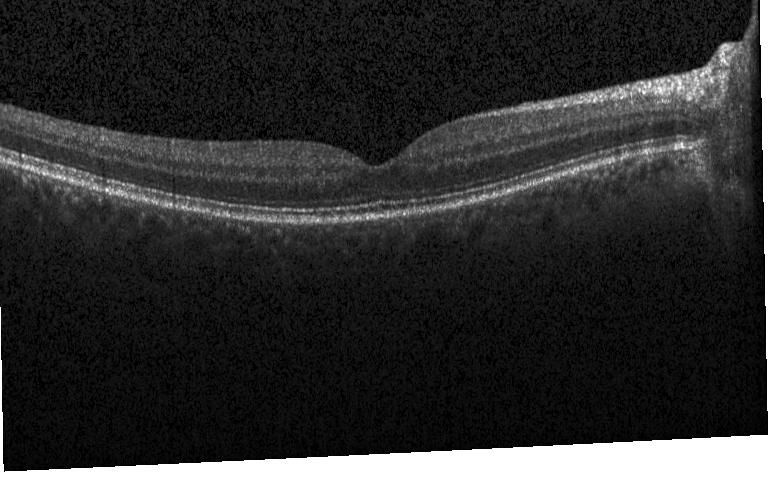 Heidelberg Spectralis, spectral-domain optical coherence tomography, OCT line scan, through the macula.
Macular OCT: no evidence of CNV, DME, or drusen.